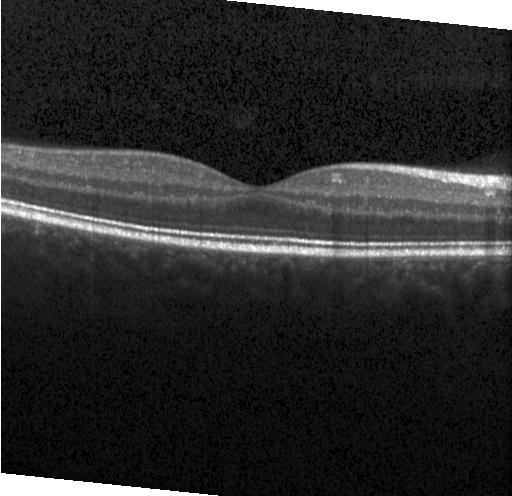
Optical coherence tomography scan. Heidelberg Spectralis OCT system. Spectral-domain OCT. Centered on the fovea
Diagnosis: no choroidal neovascularization, diabetic macular edema, or drusen.